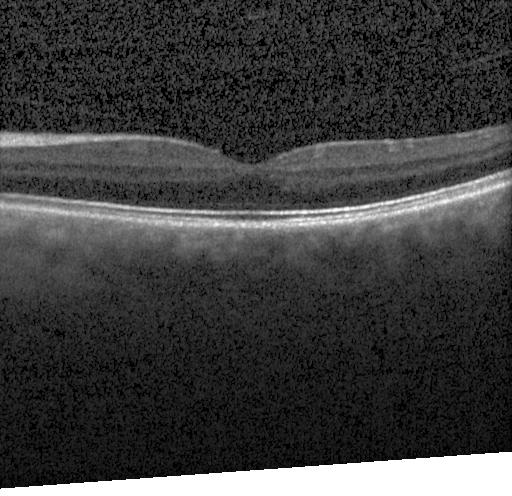
OCT line scan.
Impression: no evidence of CNV, DME, or drusen.